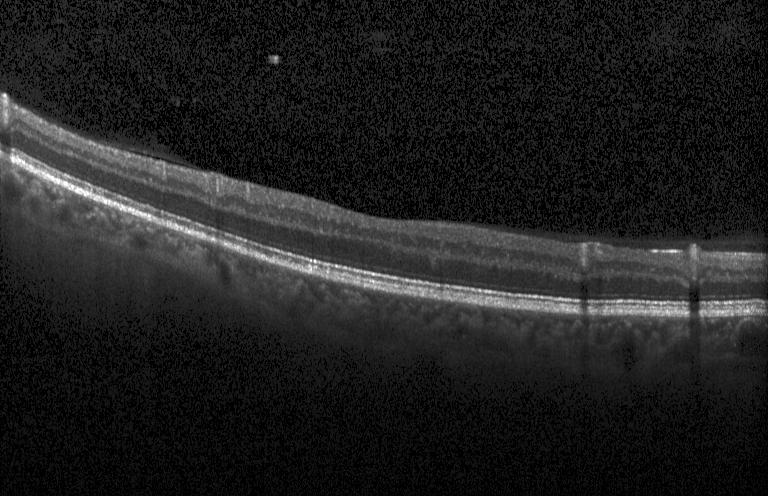
Finding: no evidence of choroidal neovascularization, diabetic macular edema, or drusen.